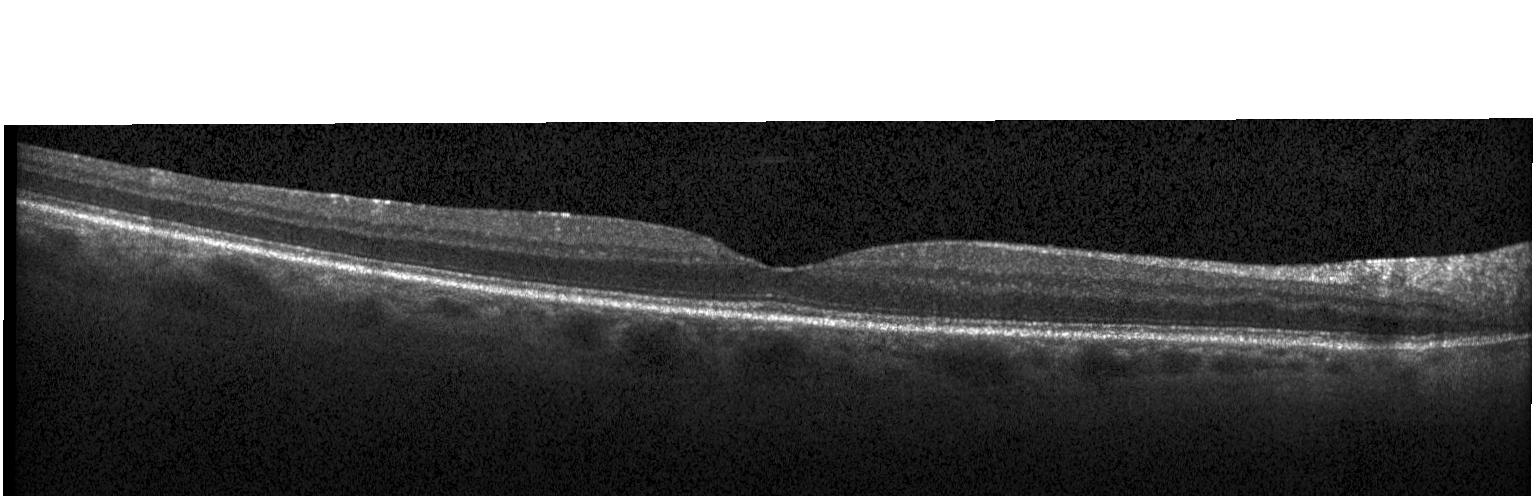
Acquired on a Heidelberg Spectralis, fovea-centered, retinal OCT cross-section, spectral-domain optical coherence tomography
Impression: no choroidal neovascularization, diabetic macular edema, or drusen.